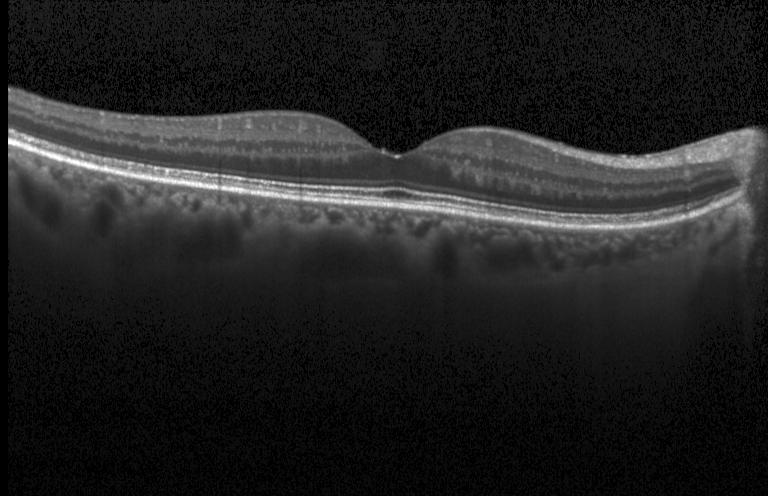

Diagnosis: no choroidal neovascularization, diabetic macular edema, or drusen.